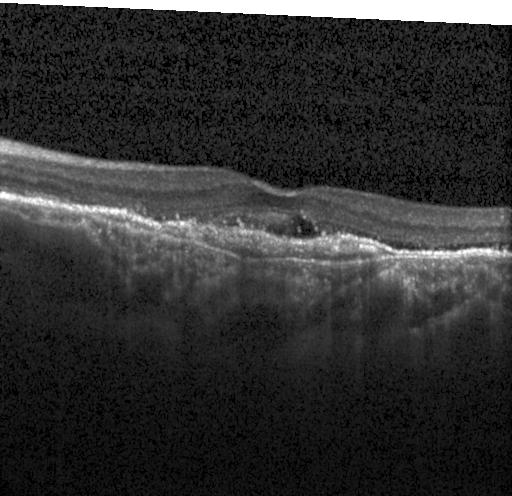
OCT scan showing choroidal neovascularization (CNV).